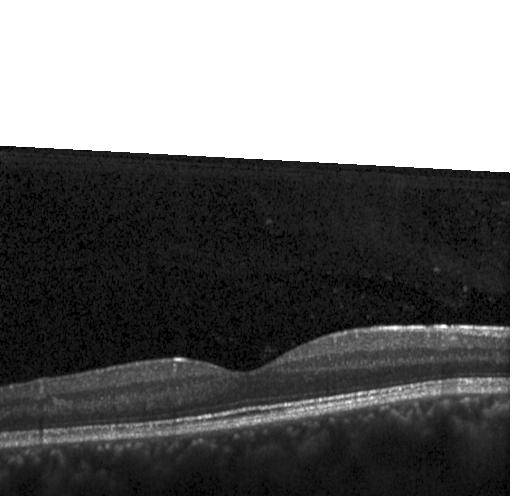

Heidelberg Spectralis. Spectral-domain optical coherence tomography. OCT B-scan. Fovea-centered — Diagnosis: no CNV, no DME, and no drusen.